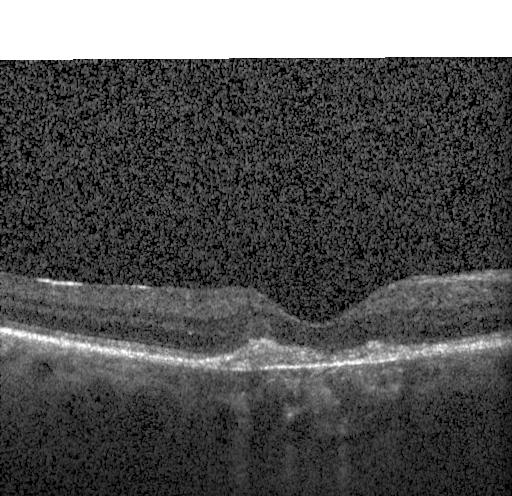
OCT line scan · SD-OCT · centered on the fovea.
This B-scan demonstrates a choroidal neovascular membrane.